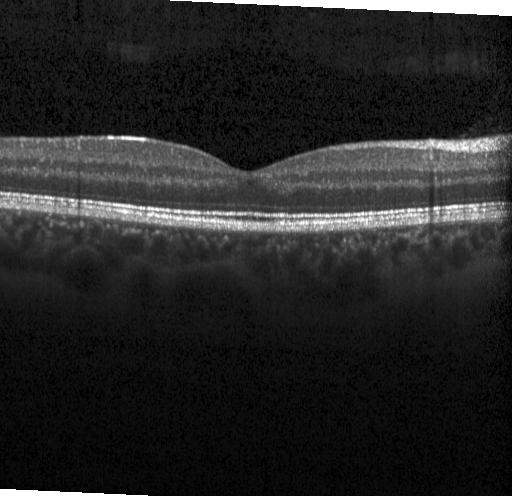

OCT line scan, horizontal scan through the fovea.
Diagnosis: neither choroidal neovascularization, diabetic macular edema, nor drusen.